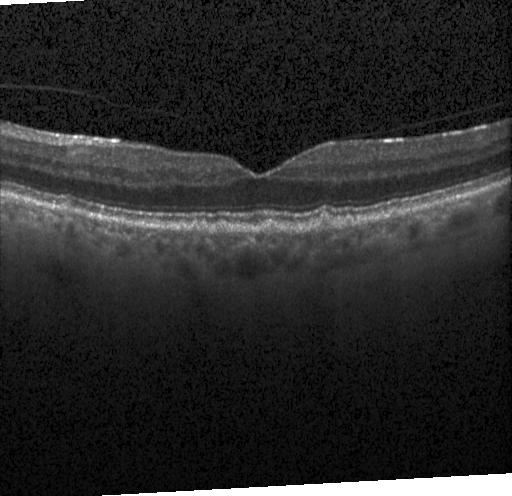
Acquired on a Heidelberg Spectralis; retinal OCT B-scan; SD-OCT.
Impression: sub-RPE drusenoid deposits.